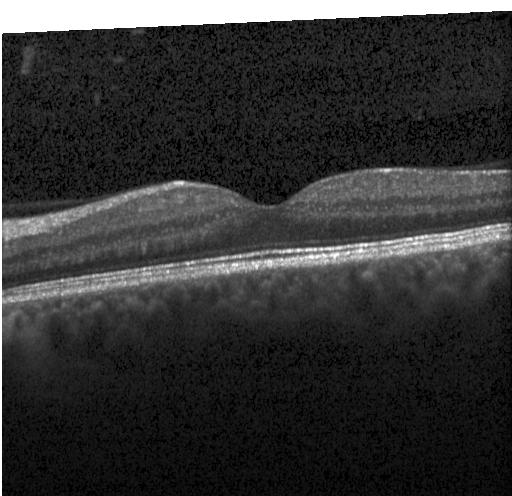

Acquired on a Heidelberg Spectralis. Optical coherence tomography B-scan. No CNV, no DME, and no drusen.